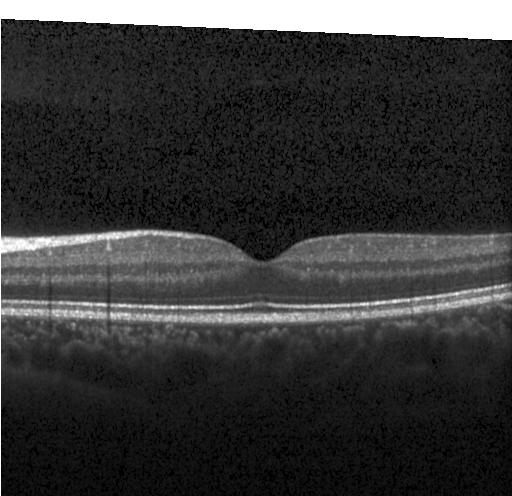
Heidelberg Spectralis. Spectral-domain OCT. OCT line scan.
Neither CNV, DME, nor drusen.